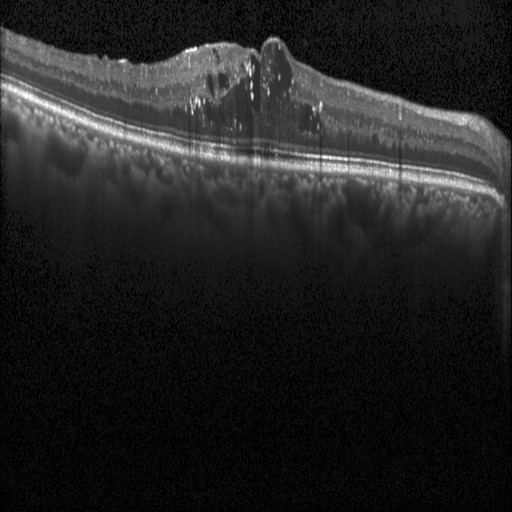 Centered on the fovea · retinal OCT cross-section · SD-OCT — This B-scan demonstrates DME.